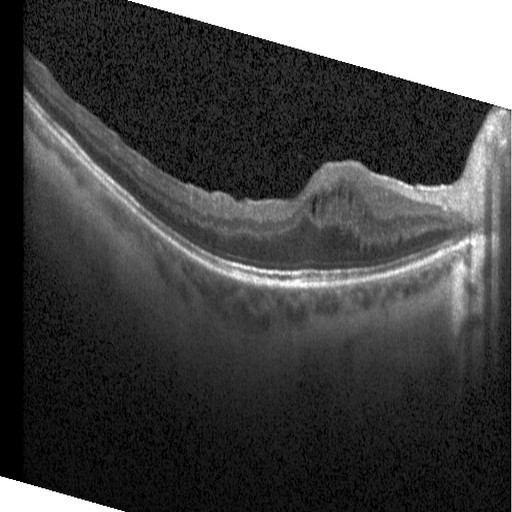

Diagnosis: diabetic macular edema.